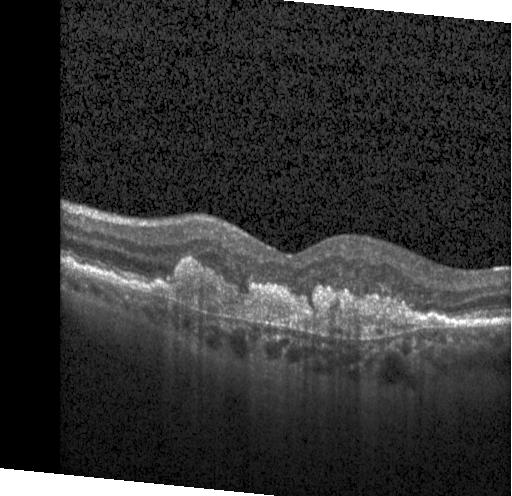 Optical coherence tomography B-scan · Heidelberg Spectralis · macular scan · SD-OCT. This B-scan demonstrates a choroidal neovascular membrane.